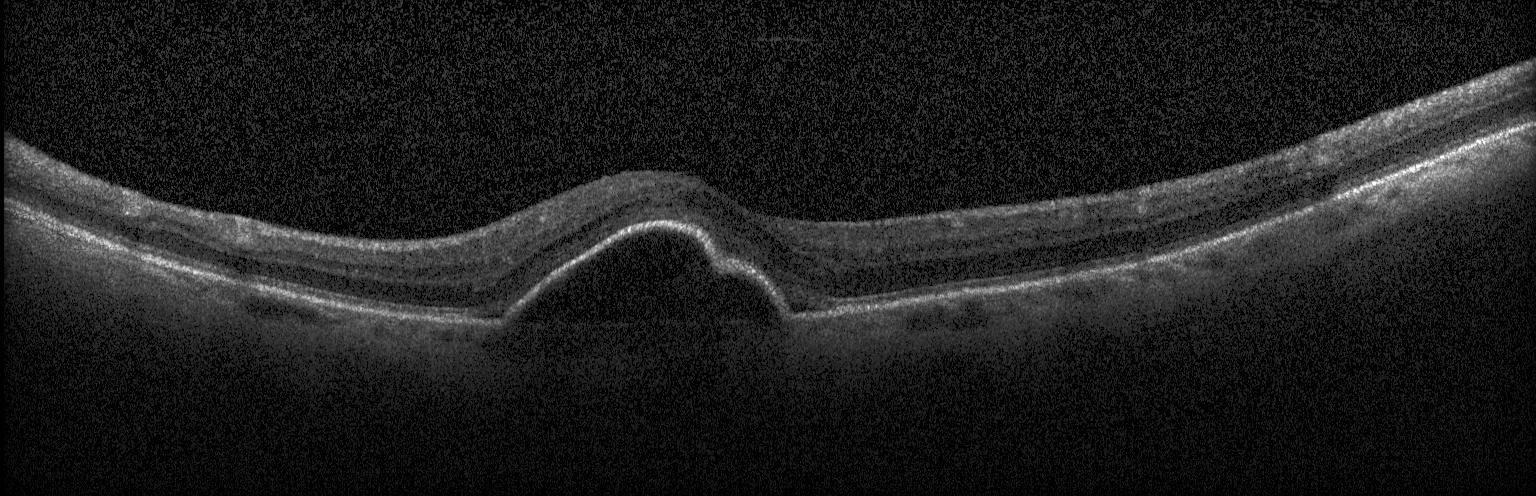
Impression: a choroidal neovascular membrane.